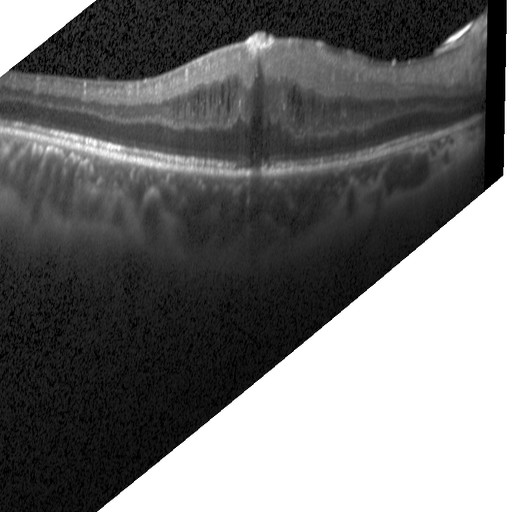 Instrument: Heidelberg Spectralis. Optical coherence tomography scan
Diagnosis: DME.